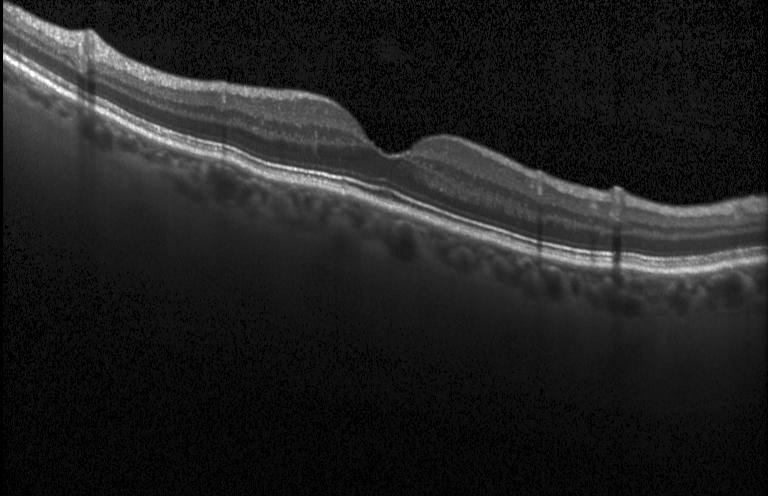 Retinal OCT cross-section showing neither CNV, DME, nor drusen.